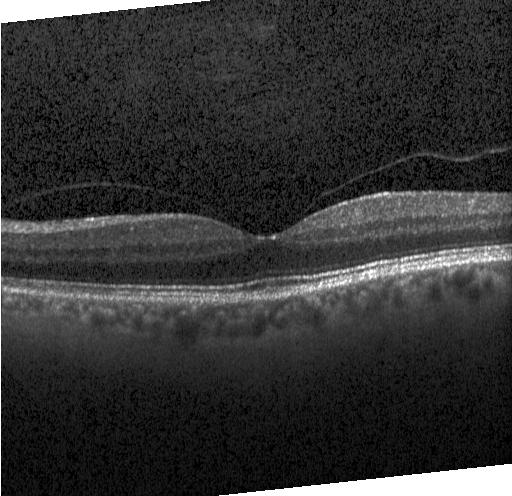

OCT B-scan. Finding: no choroidal neovascularization, no diabetic macular edema, and no drusen.